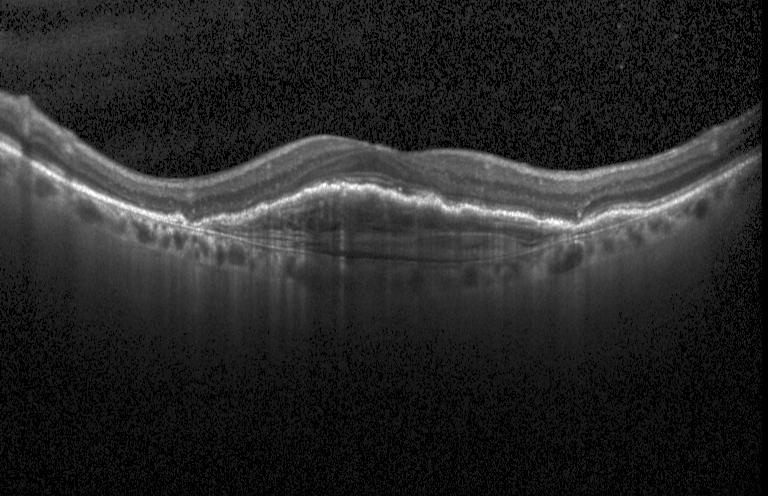

Macular OCT demonstrating CNV.